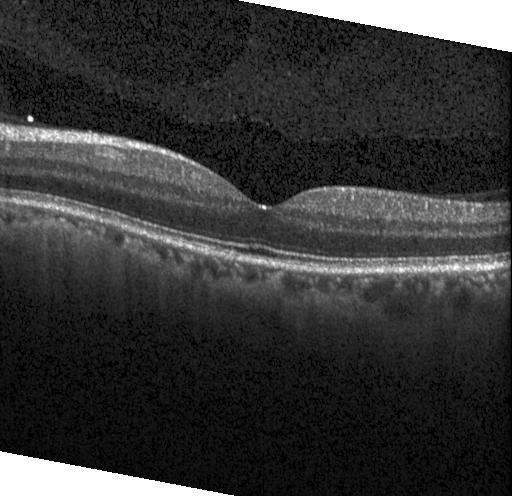

SD-OCT; OCT B-scan.
No choroidal neovascularization, no diabetic macular edema, and no drusen.